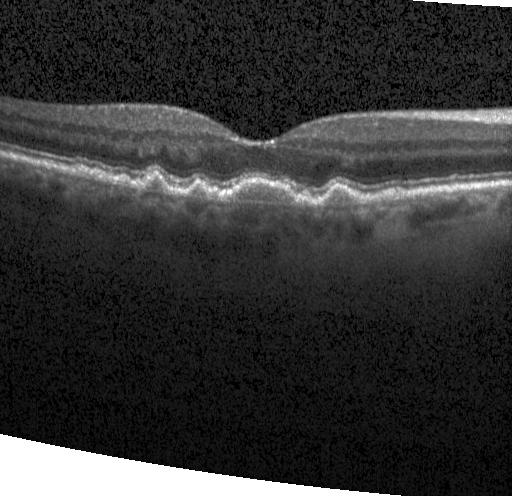 Macular OCT demonstrating multiple drusen.